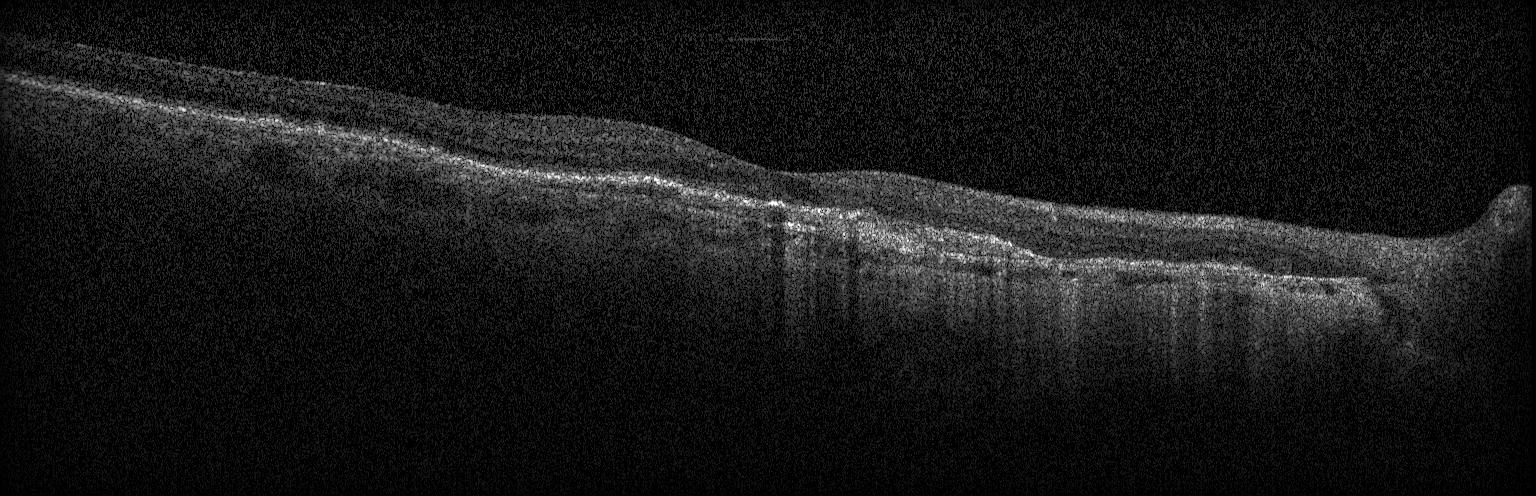
OCT B-scan. Through the macula.
Assessment: CNV.